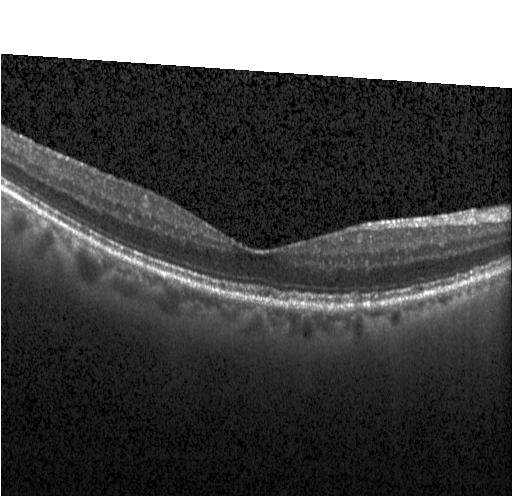
OCT B-scan — Assessment: drusen.